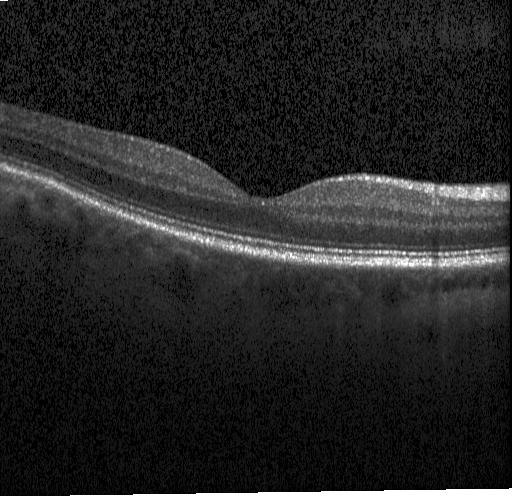 Diagnosis: no CNV, DME, or drusen.